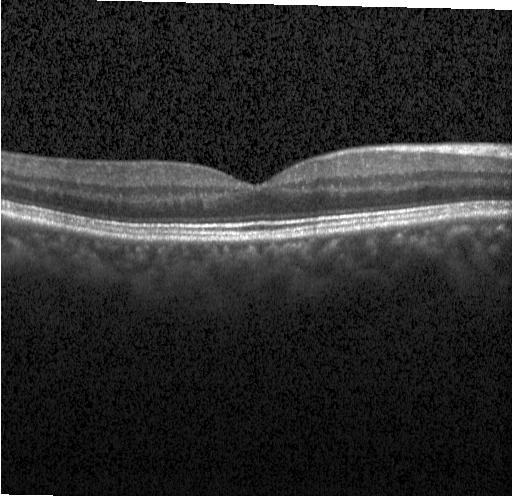 OCT B-scan showing no CNV, no DME, and no drusen.